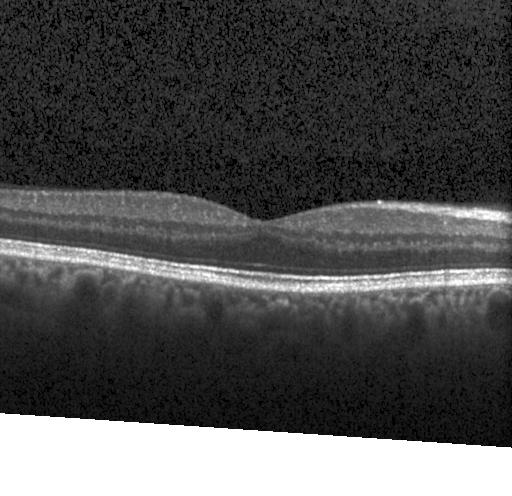

Finding: no choroidal neovascularization, no diabetic macular edema, and no drusen.